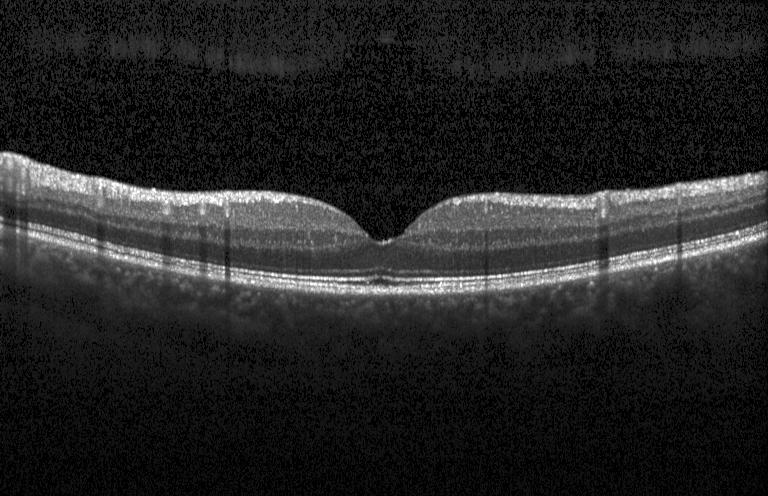 Spectral-domain OCT B-scan: neither CNV, DME, nor drusen.